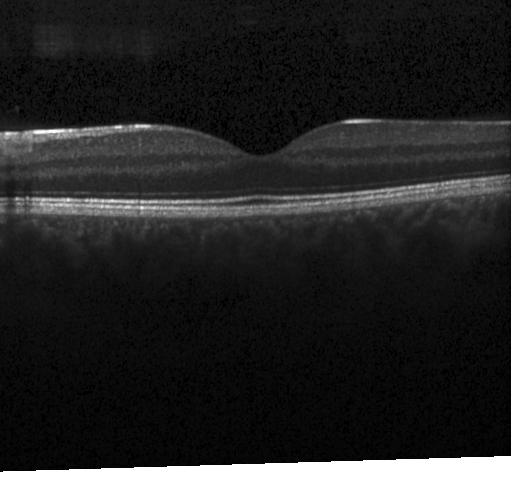 Centered on the fovea. Acquired on a Heidelberg Spectralis. Retinal OCT cross-section.
Dx: no evidence of choroidal neovascularization, diabetic macular edema, or drusen.